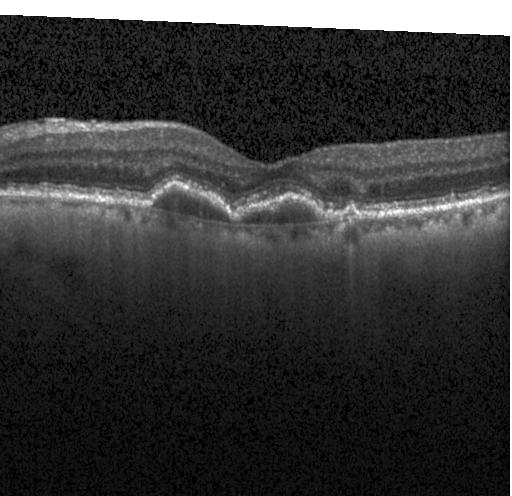

Spectral-domain OCT. OCT B-scan. Instrument: Heidelberg Spectralis — Dx: choroidal neovascularization (CNV).